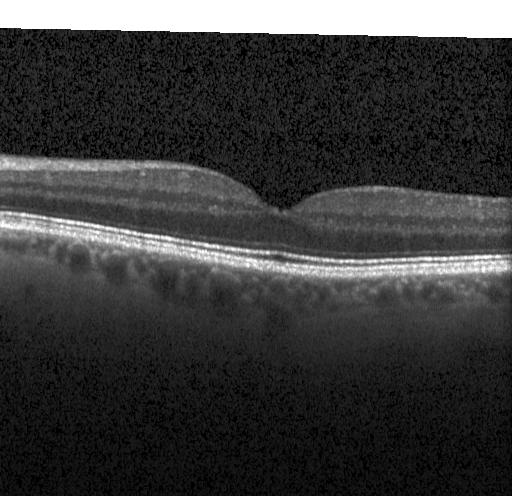

Spectral-domain optical coherence tomography; OCT line scan; fovea-centered; Heidelberg Spectralis OCT system.
This B-scan demonstrates neither choroidal neovascularization, diabetic macular edema, nor drusen.